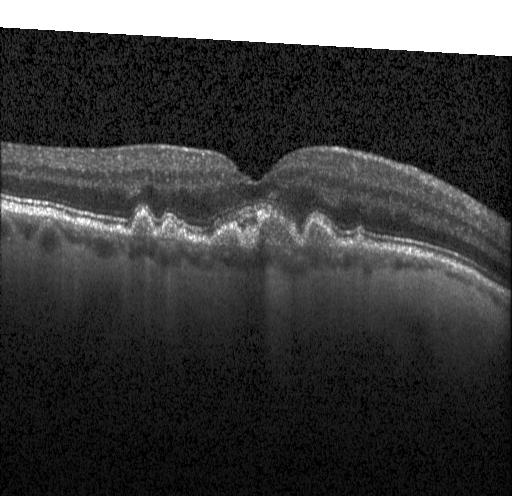 Acquired on a Heidelberg Spectralis · macular scan · optical coherence tomography B-scan
Assessment: multiple drusen.